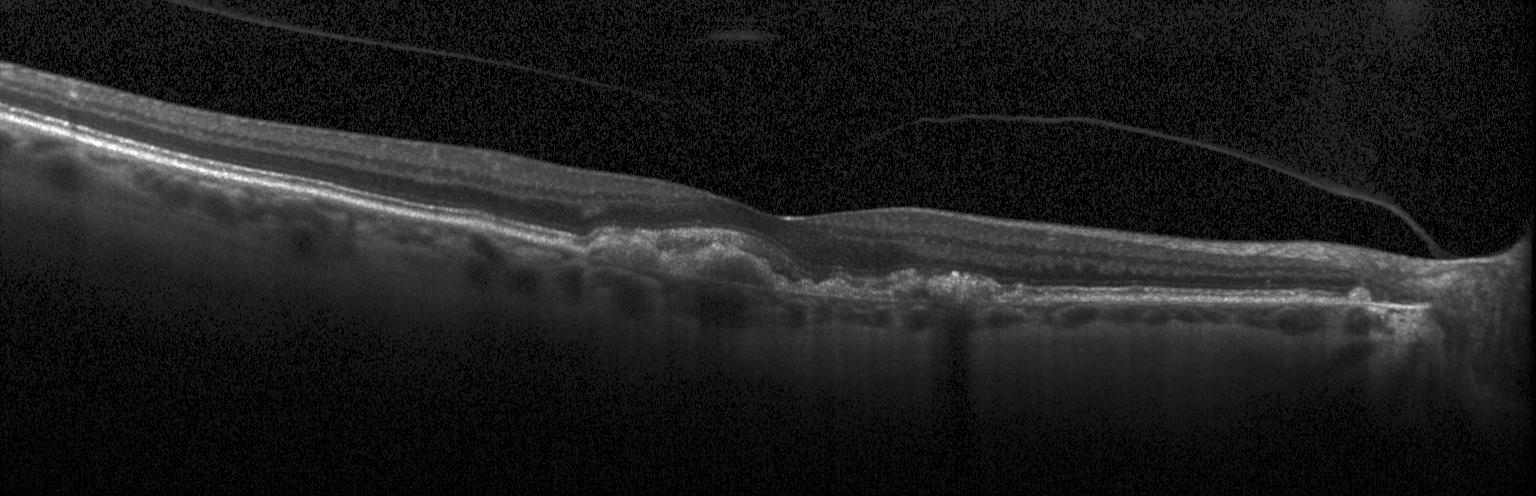 Diagnosis: a choroidal neovascular membrane.